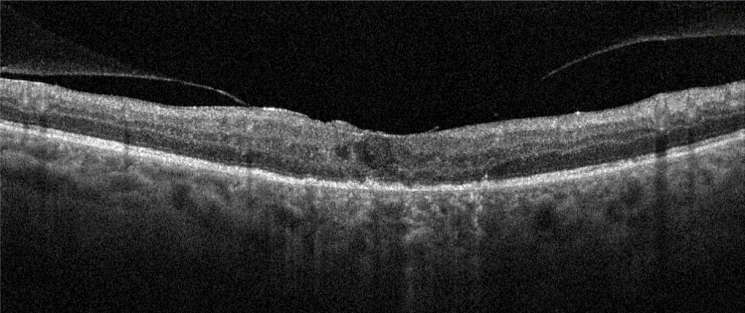 Retinal OCT B-scan, fovea-centered, Optovue Avanti RTVue XR
Macular OCT: DME.